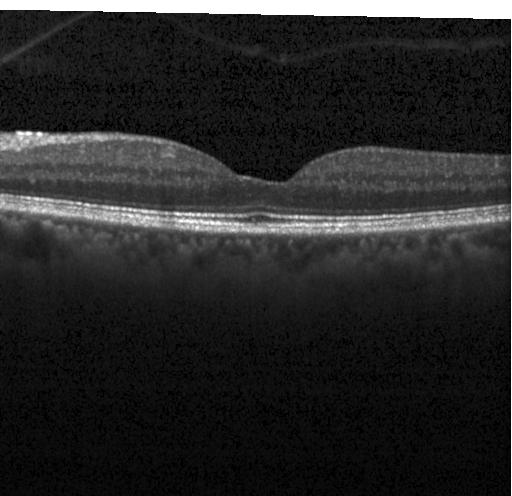

The scan shows no CNV, DME, or drusen.